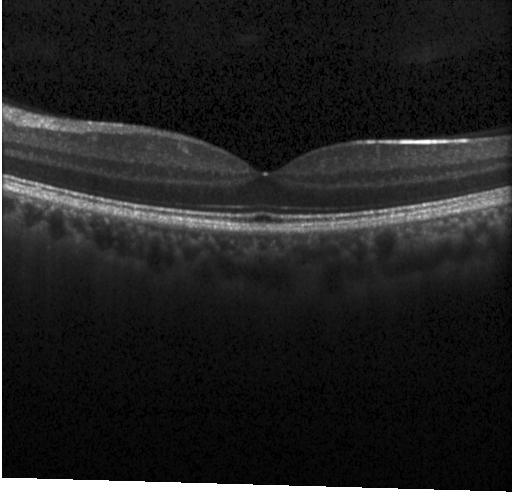
Spectral-domain optical coherence tomography · fovea-centered · optical coherence tomography scan · Heidelberg Spectralis — This B-scan demonstrates no CNV, no DME, and no drusen.